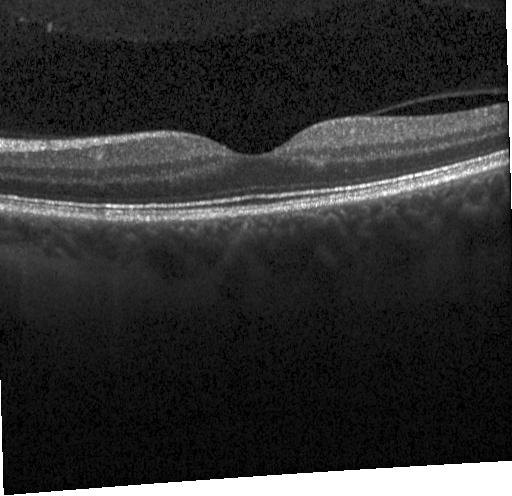
Horizontal scan through the fovea, SD-OCT, optical coherence tomography scan, instrument: Heidelberg Spectralis. Assessment: no CNV, DME, or drusen.